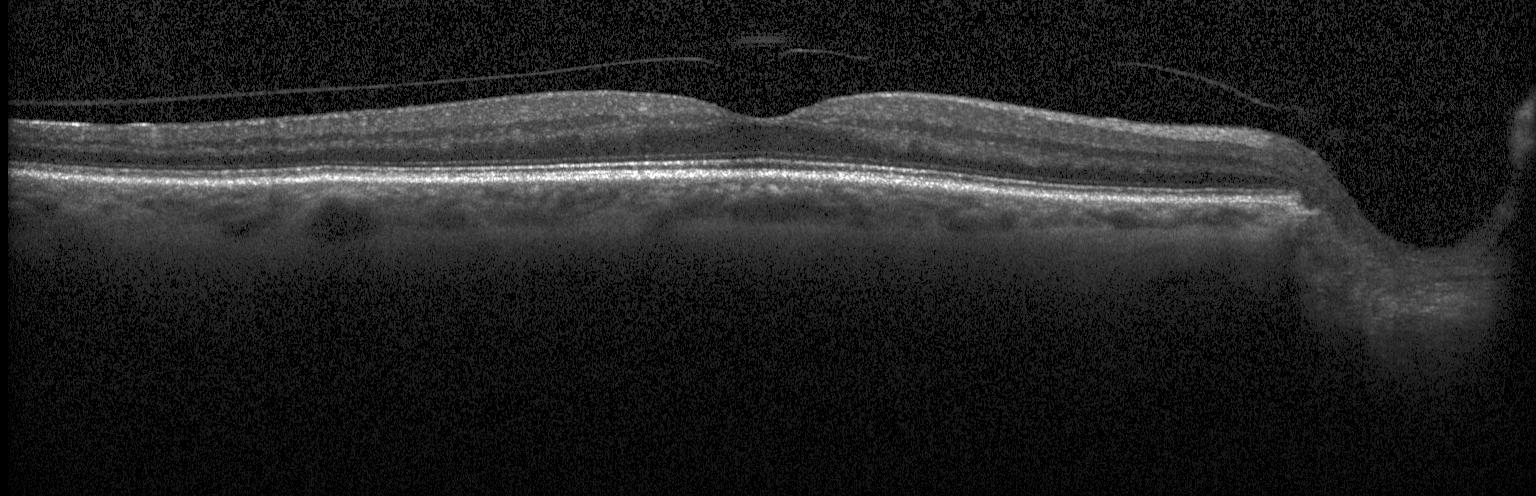 Heidelberg Spectralis OCT system, horizontal scan through the fovea, optical coherence tomography scan, SD-OCT.
Impression: no choroidal neovascularization, no diabetic macular edema, and no drusen.